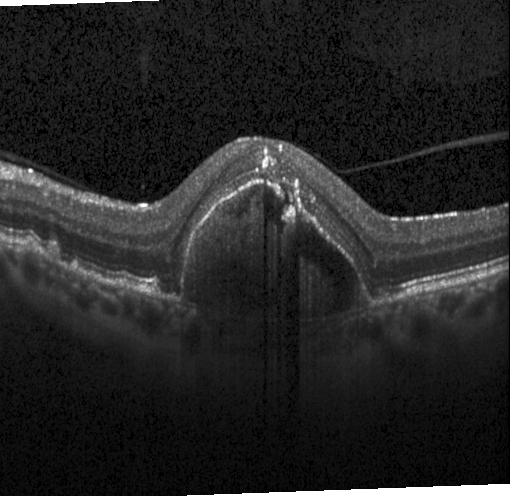
Instrument: Heidelberg Spectralis; OCT line scan — Finding: CNV.